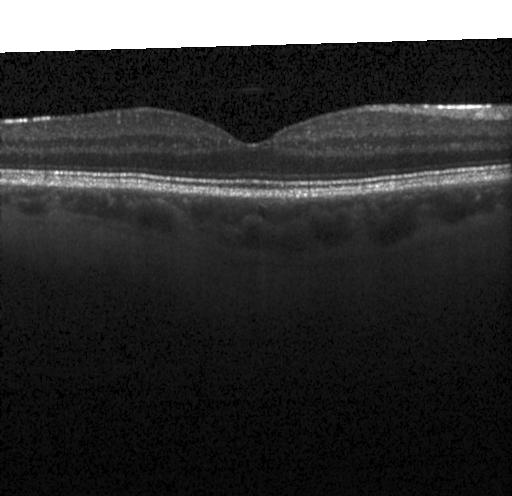

OCT line scan — OCT finding: no evidence of choroidal neovascularization, diabetic macular edema, or drusen.